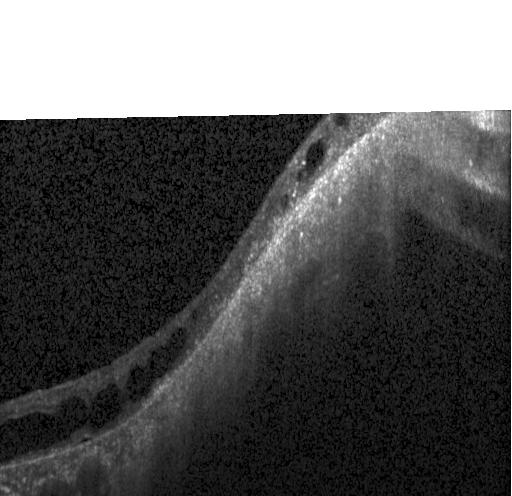

Spectral-domain OCT, retinal OCT B-scan
Impression: DME.